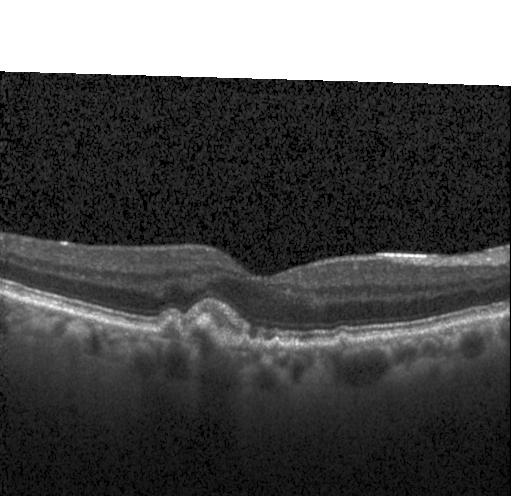

Dx: a choroidal neovascular membrane.